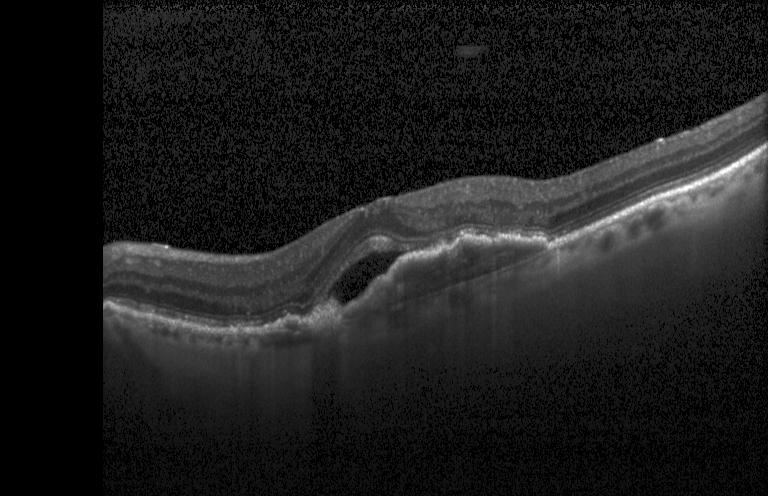 Acquired on a Heidelberg Spectralis · spectral-domain OCT · optical coherence tomography scan.
The scan shows a choroidal neovascular membrane.